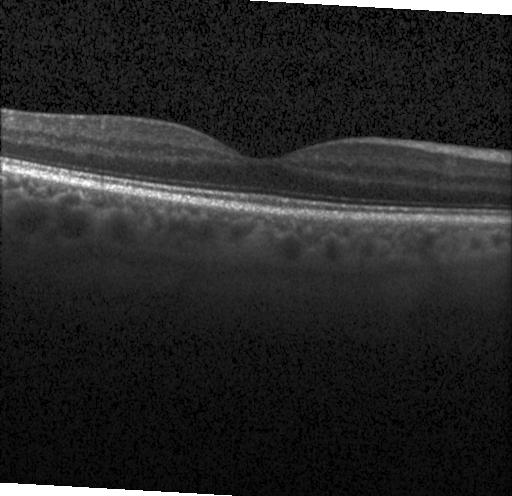 OCT finding: no CNV, no DME, and no drusen.